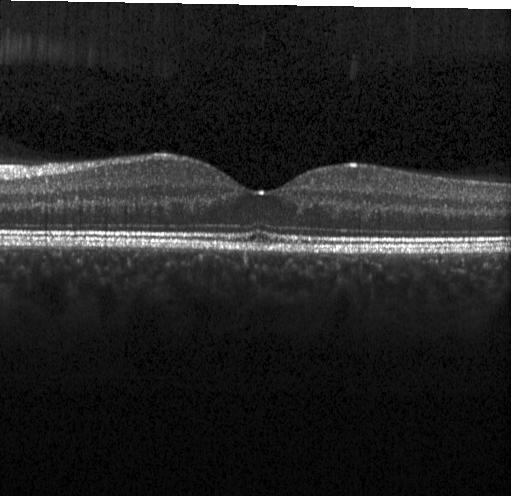
Dx: no CNV, DME, or drusen.